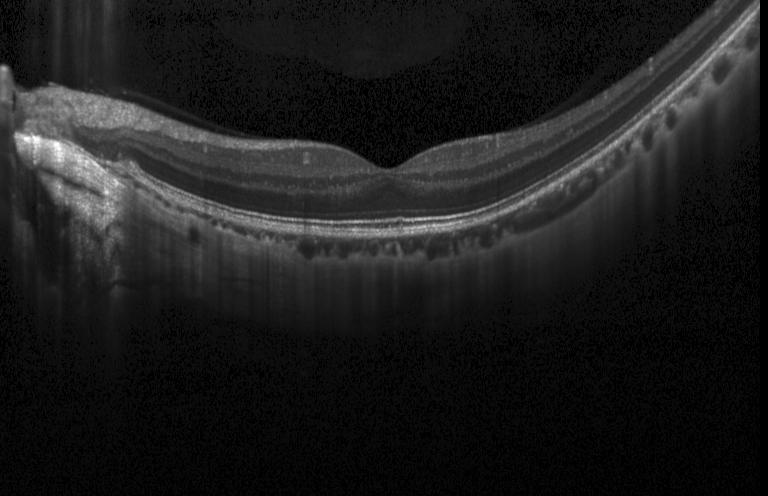 Assessment: no CNV, DME, or drusen.